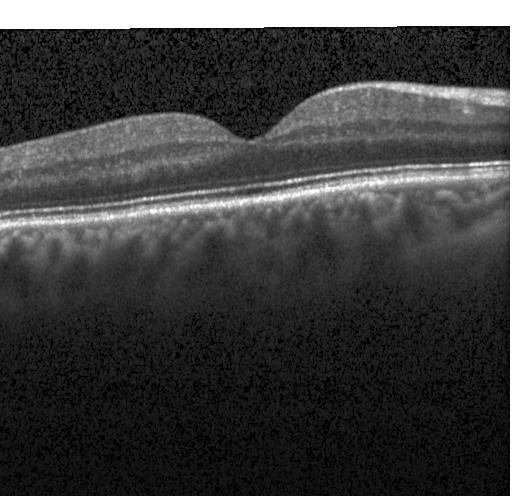
Spectral-domain OCT B-scan: no choroidal neovascularization, diabetic macular edema, or drusen.